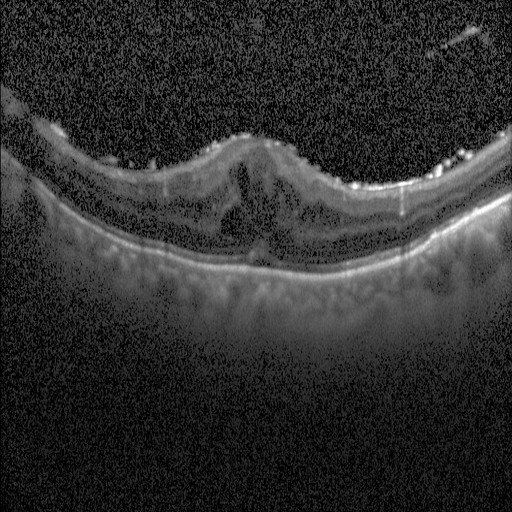

Retinal OCT B-scan. SD-OCT
Diagnosis: diabetic macular edema.